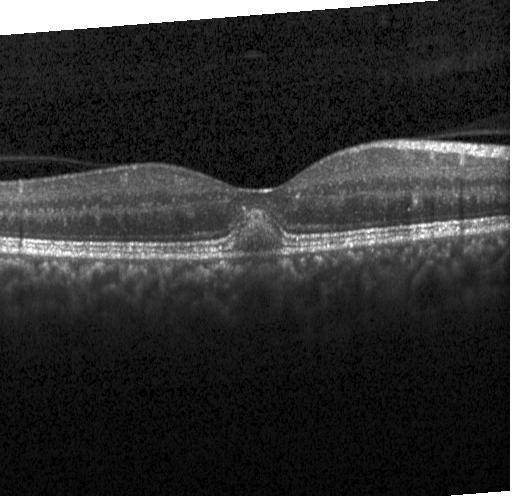

Macular OCT: a choroidal neovascular membrane.